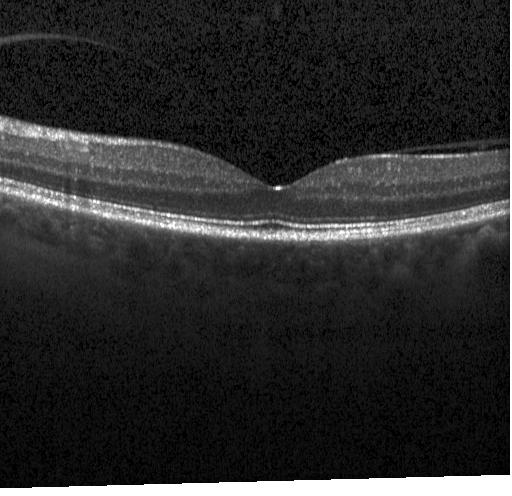
OCT line scan
The scan shows no evidence of choroidal neovascularization, diabetic macular edema, or drusen.